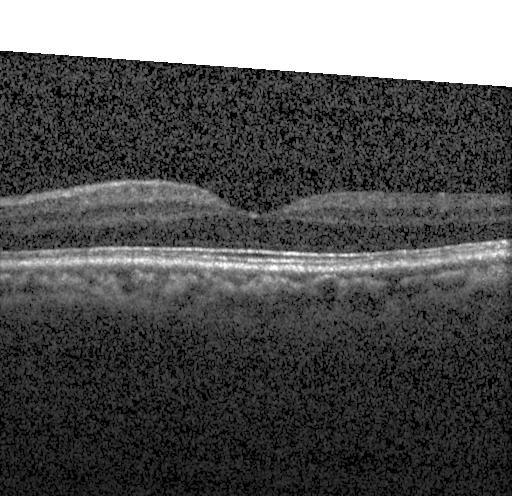 Through the macula, optical coherence tomography B-scan. Assessment: neither CNV, DME, nor drusen.